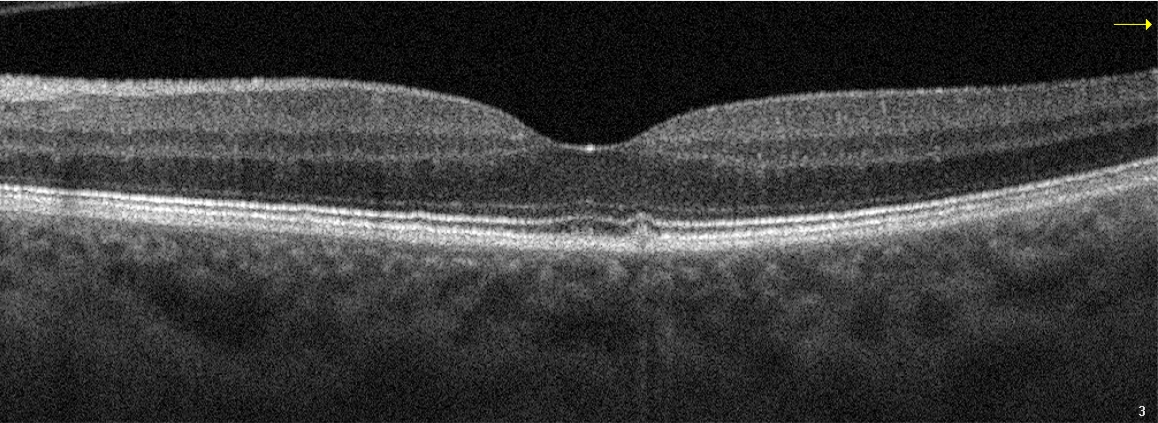

Acquired on an Optovue Avanti RTVue XR, retinal OCT cross-section, through the macula — Diagnosis: age-related macular degeneration (AMD).